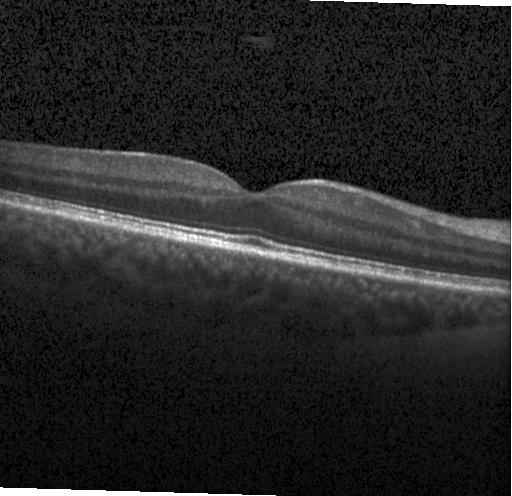

OCT B-scan.
Diagnosis: no CNV, DME, or drusen.